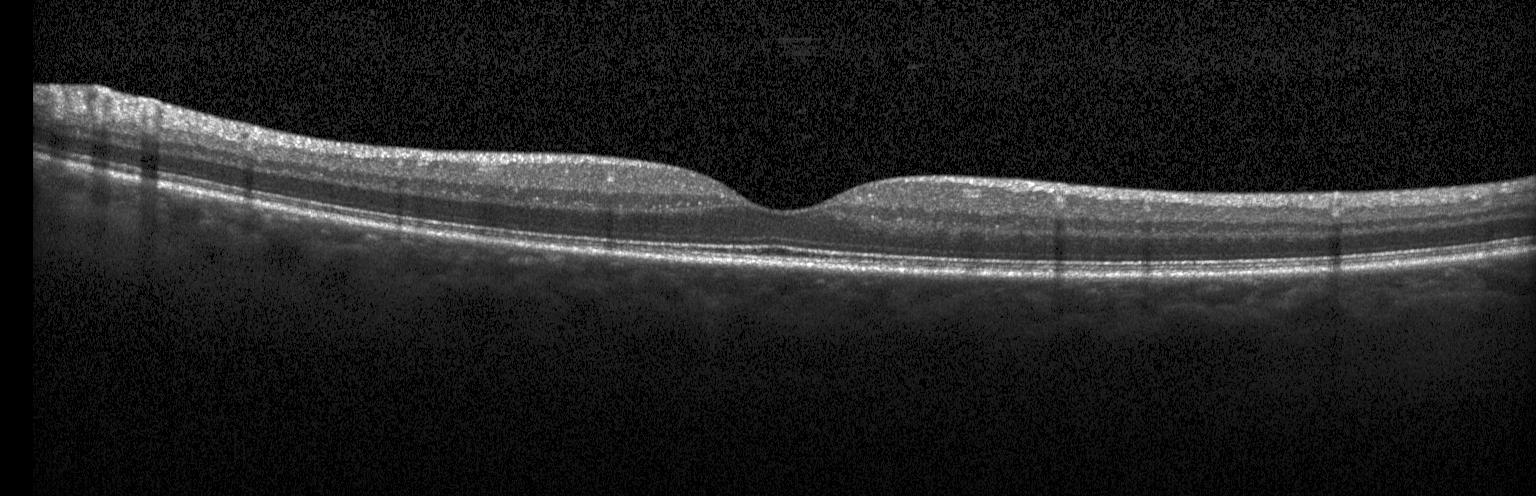 Impression: no evidence of choroidal neovascularization, diabetic macular edema, or drusen.